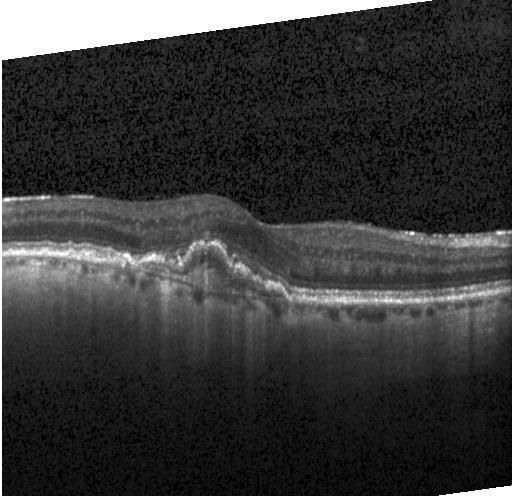
OCT B-scan — Impression: CNV.